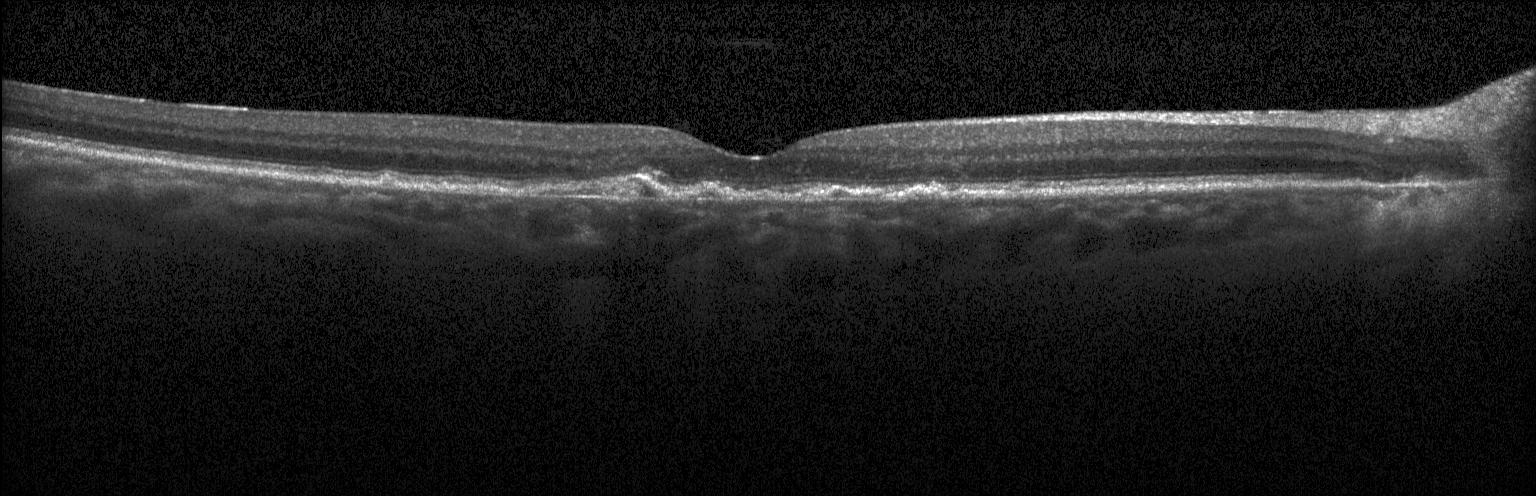 Centered on the fovea; retinal OCT B-scan; acquired on a Heidelberg Spectralis
This B-scan demonstrates CNV.